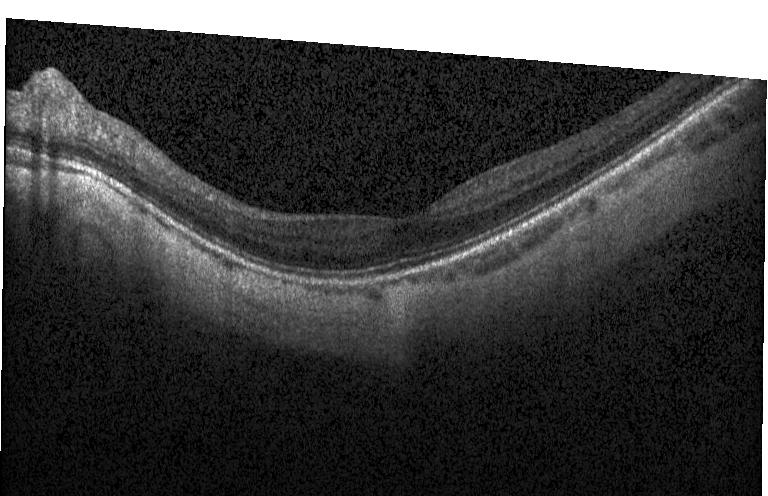
Optical coherence tomography scan · centered on the fovea · instrument: Heidelberg Spectralis — Impression: no choroidal neovascularization, no diabetic macular edema, and no drusen.